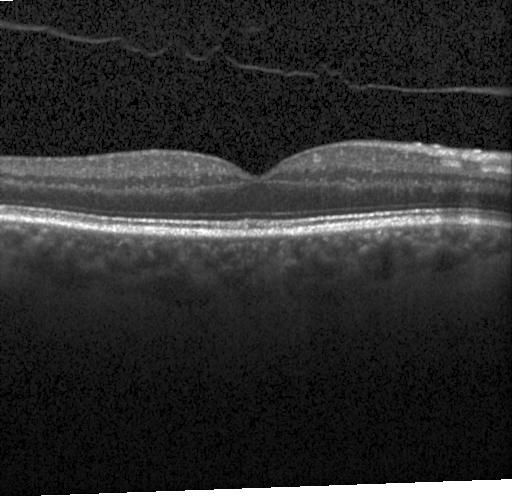 Diagnosis: no choroidal neovascularization, no diabetic macular edema, and no drusen.